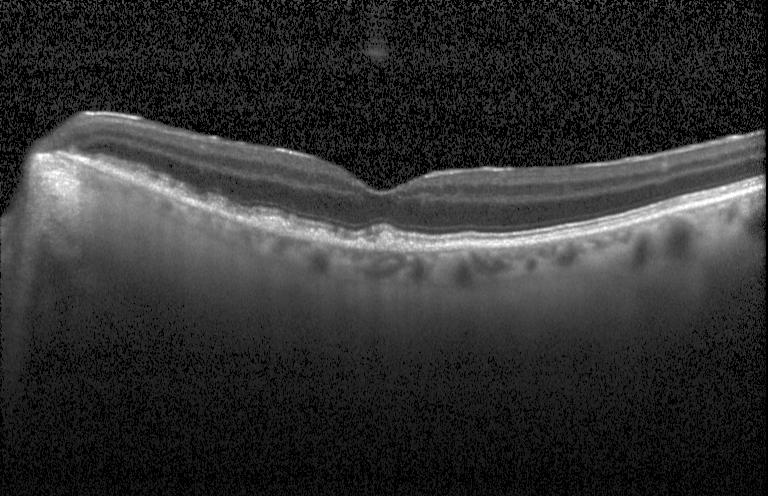

Diagnosis: sub-RPE drusenoid deposits.